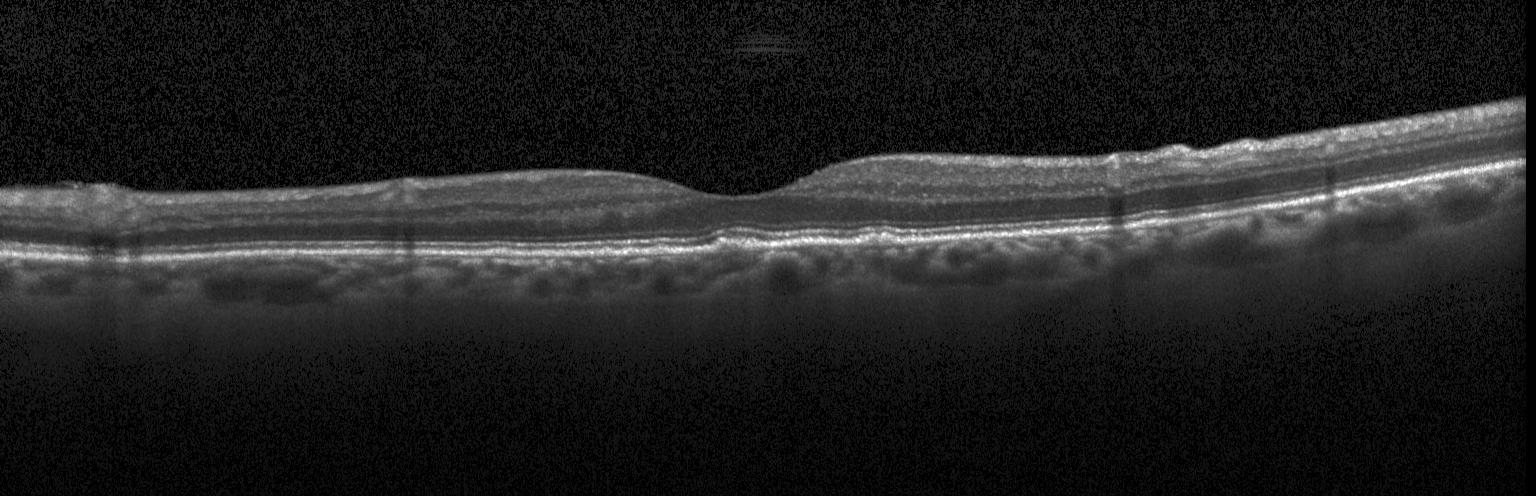
Dx: sub-RPE drusenoid deposits.